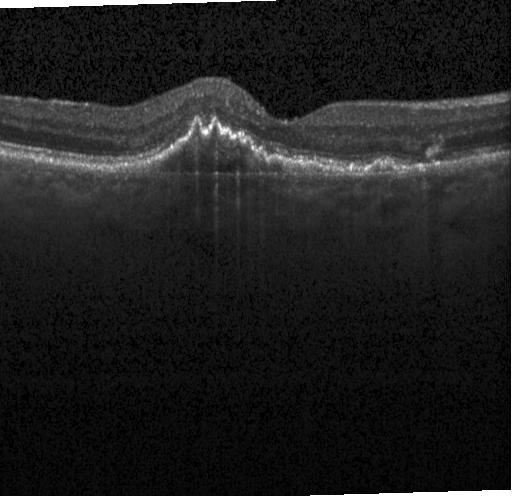
OCT B-scan showing a choroidal neovascular membrane.